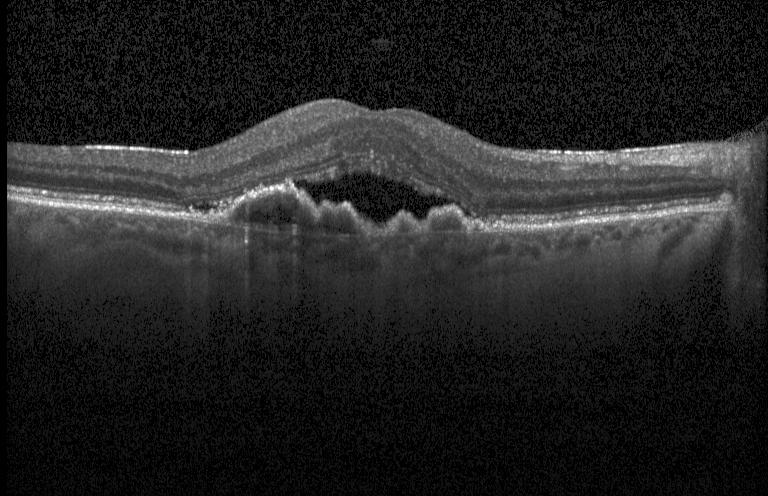

Retinal OCT cross-section showing a choroidal neovascular membrane.